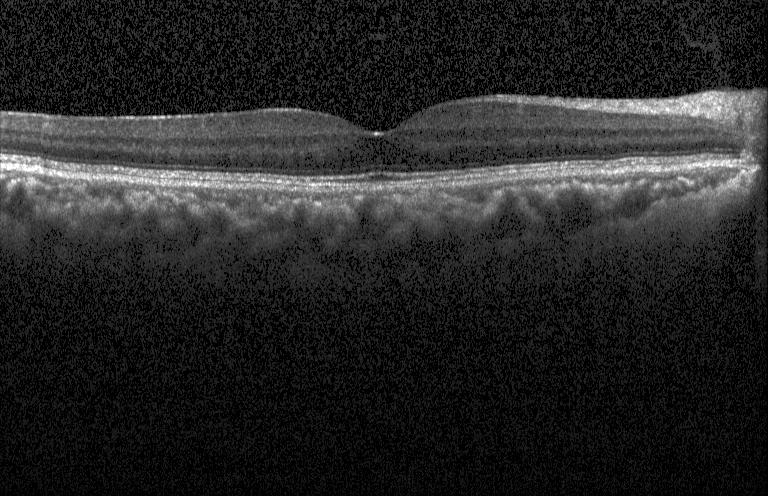 Heidelberg Spectralis OCT system. Retinal OCT cross-section
This B-scan demonstrates no CNV, no DME, and no drusen.